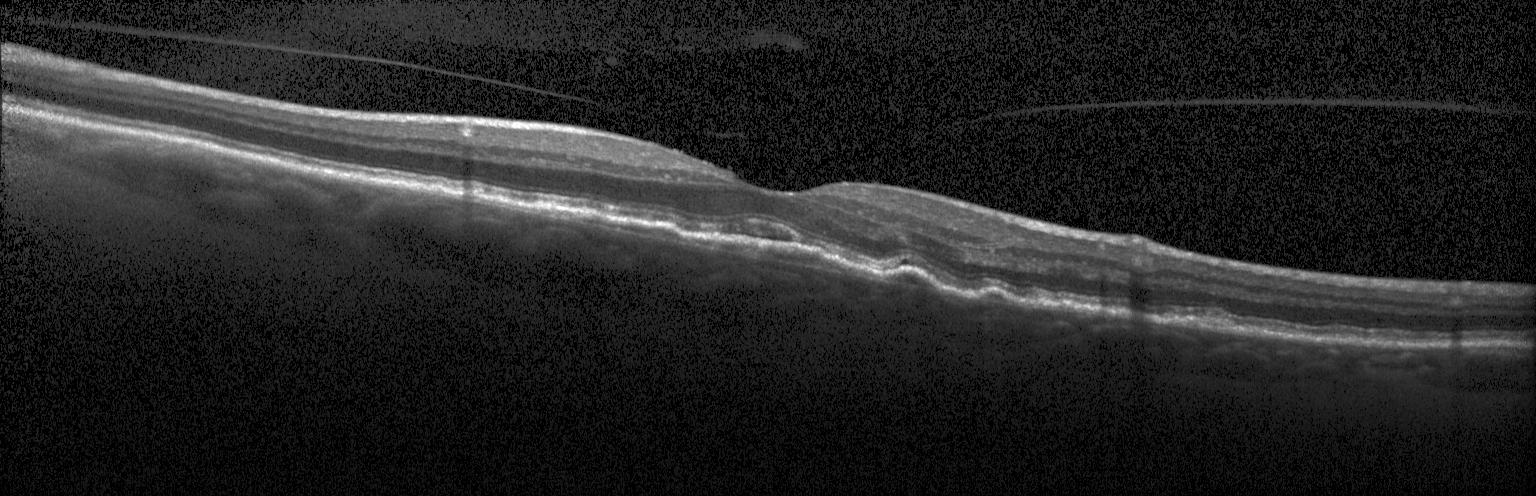 OCT B-scan.
The scan shows CNV.